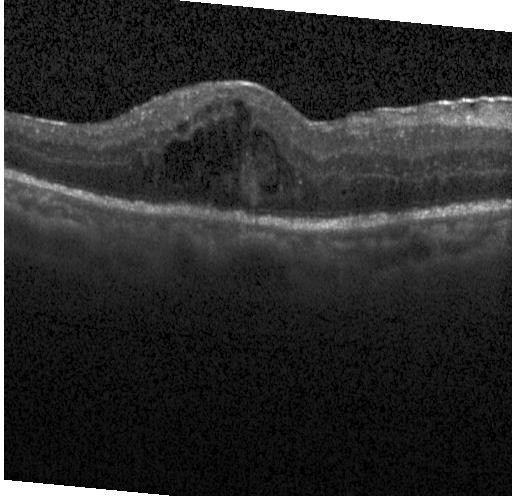
OCT finding: diabetic macular edema (DME).